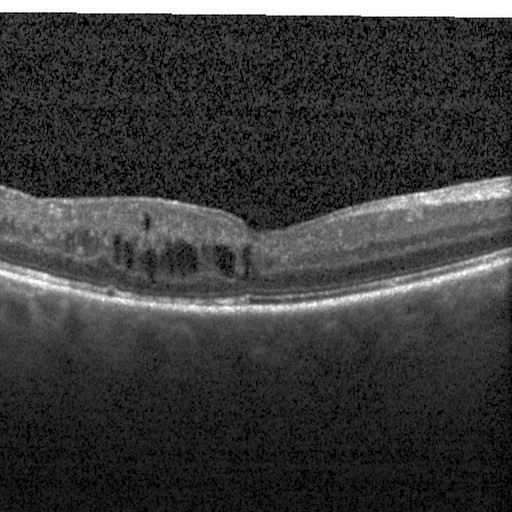 This B-scan demonstrates diabetic macular edema.